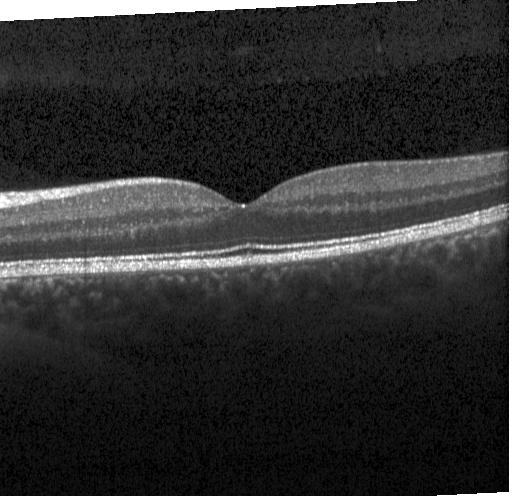
Diagnosis: no evidence of CNV, DME, or drusen.